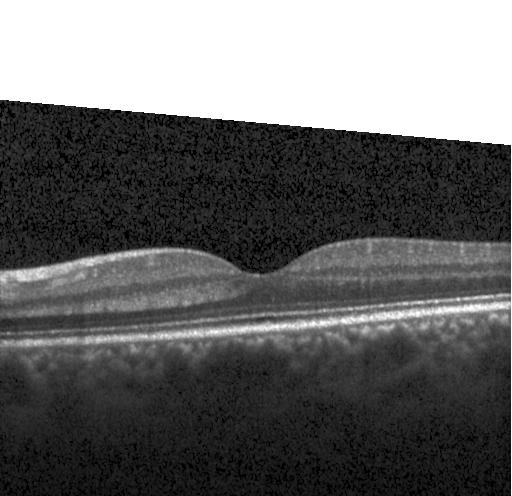 OCT line scan; SD-OCT — Finding: no evidence of choroidal neovascularization, diabetic macular edema, or drusen.